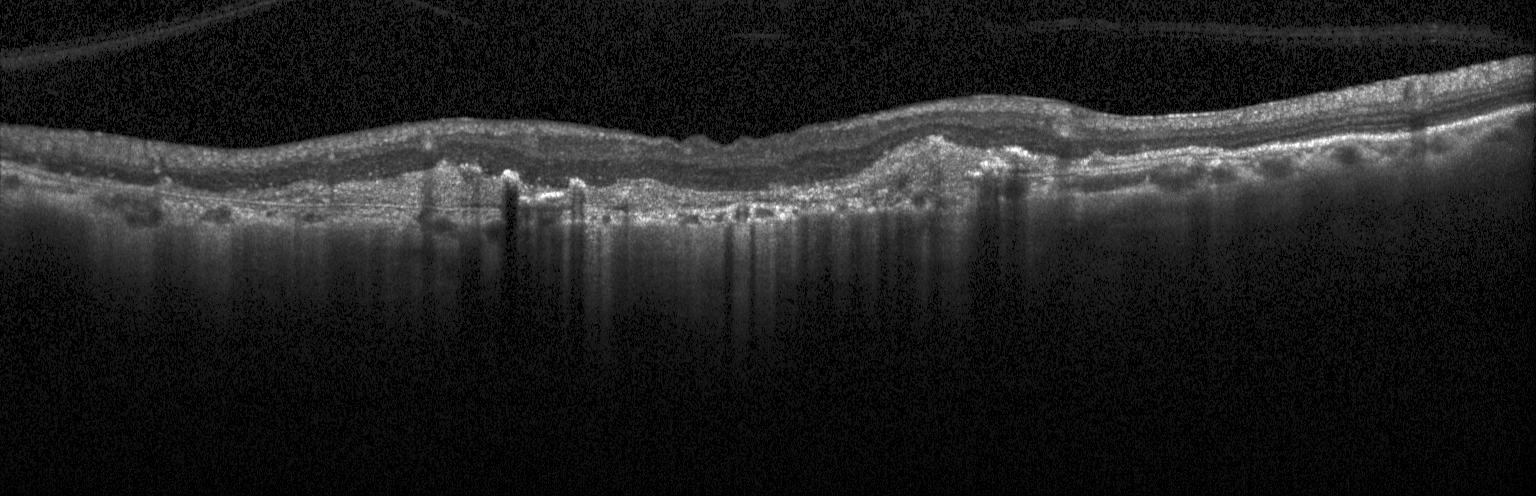
Retinal OCT cross-section.
Assessment: CNV.